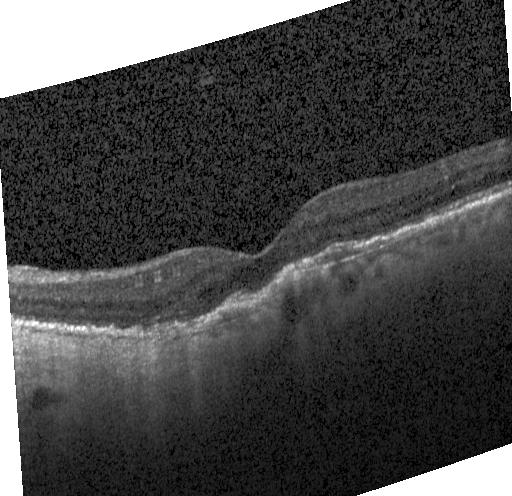
Optical coherence tomography scan
Finding: a choroidal neovascular membrane.